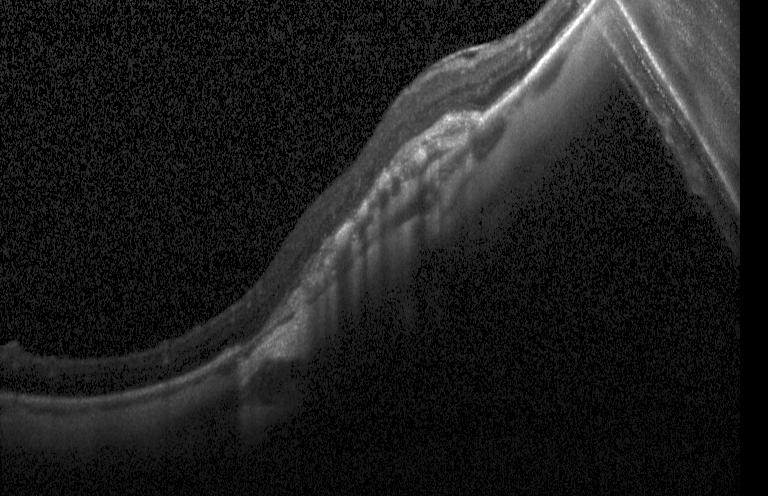

A choroidal neovascular membrane.